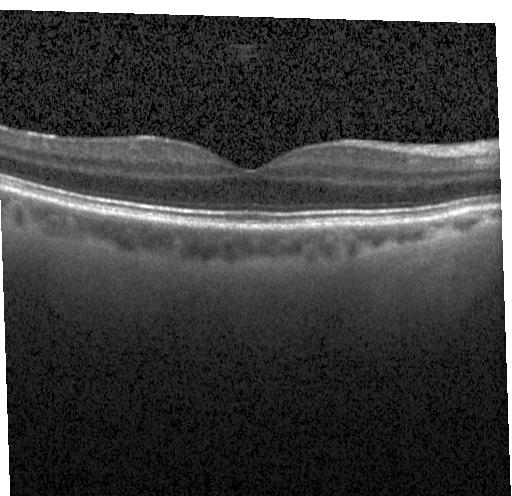

Finding: no choroidal neovascularization, no diabetic macular edema, and no drusen.